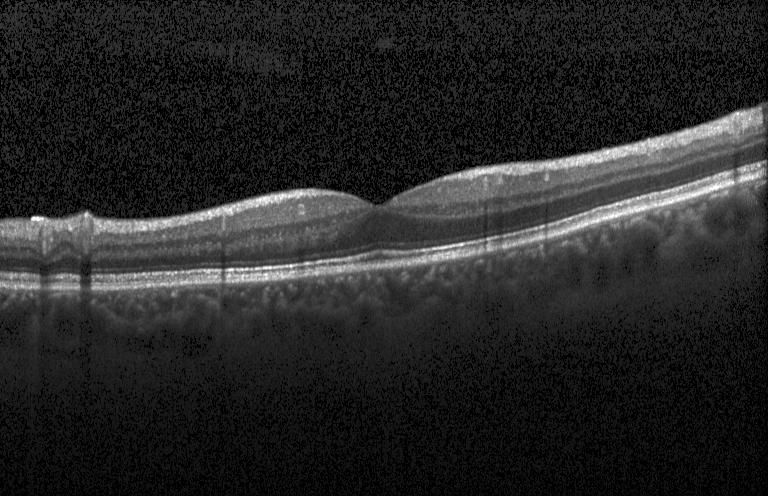
Finding: no CNV, DME, or drusen.